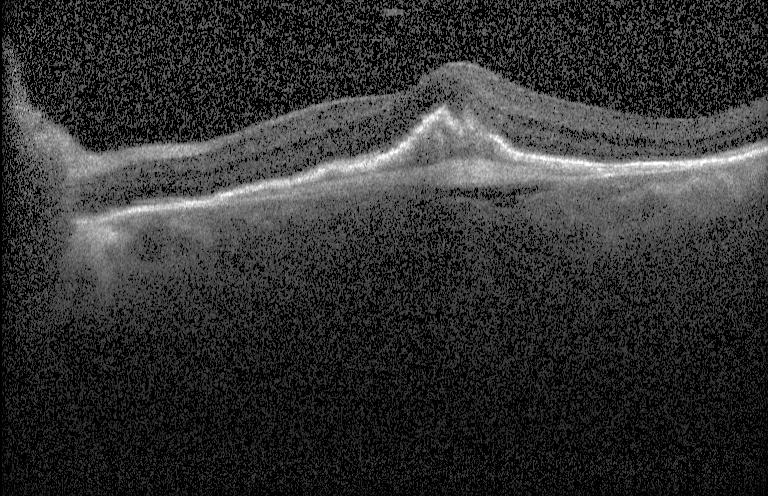

Retinal OCT cross-section. Macular OCT: a choroidal neovascular membrane.